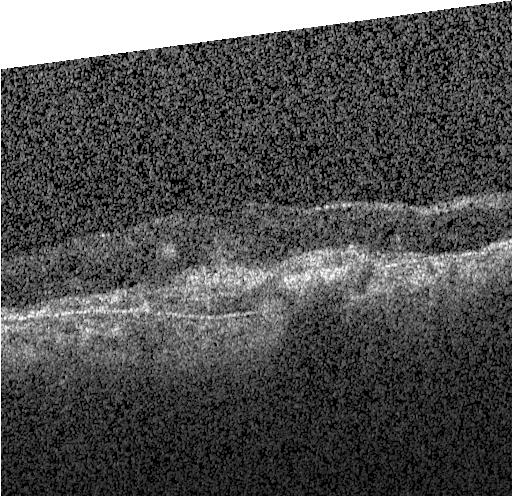 OCT B-scan. Impression: choroidal neovascularization.